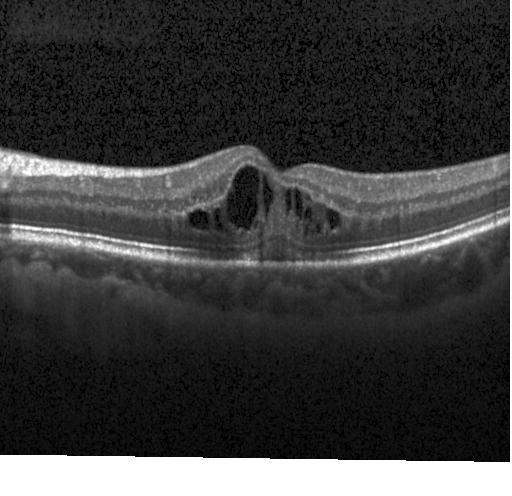 This B-scan demonstrates diabetic macular edema (DME).